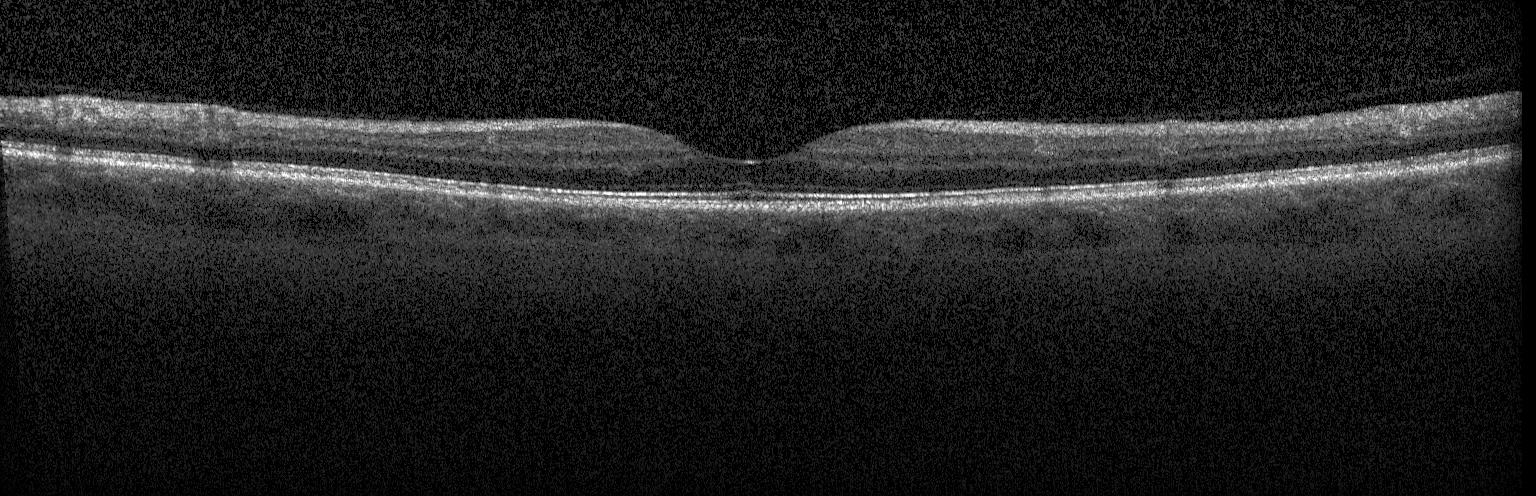 Diagnosis: no CNV, DME, or drusen.